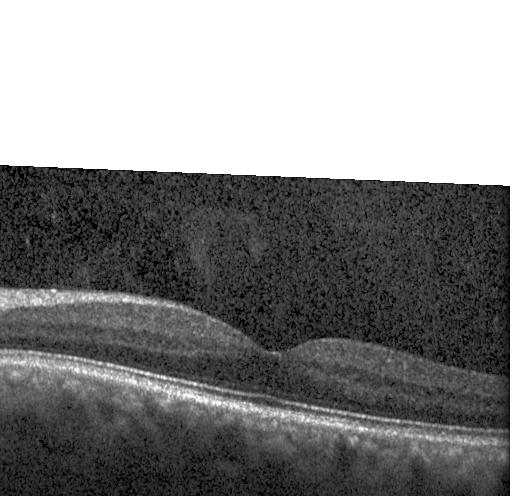
OCT B-scan, macular scan, spectral-domain OCT, instrument: Heidelberg Spectralis
This B-scan demonstrates no choroidal neovascularization, diabetic macular edema, or drusen.